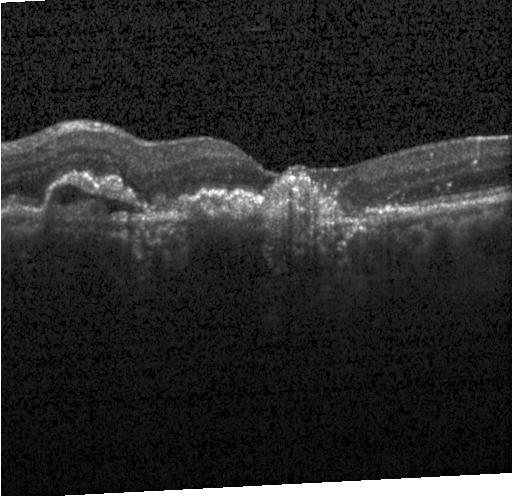

Finding: choroidal neovascularization (CNV).